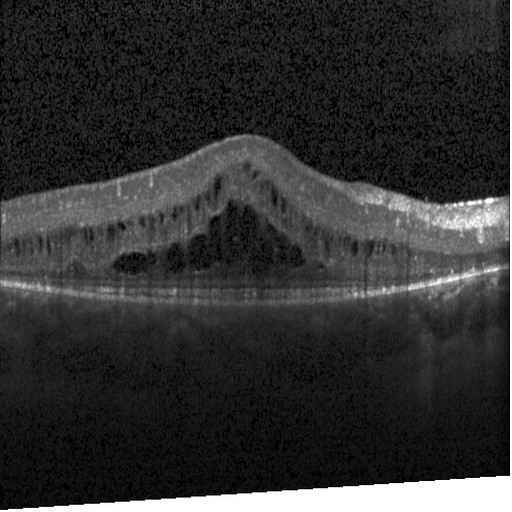
Impression: diabetic macular edema.